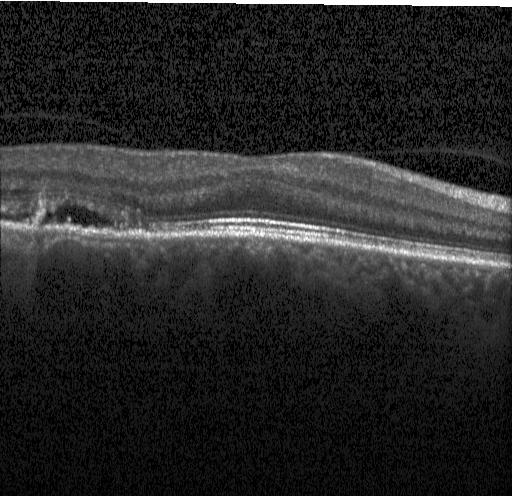

Macular OCT demonstrating a choroidal neovascular membrane.